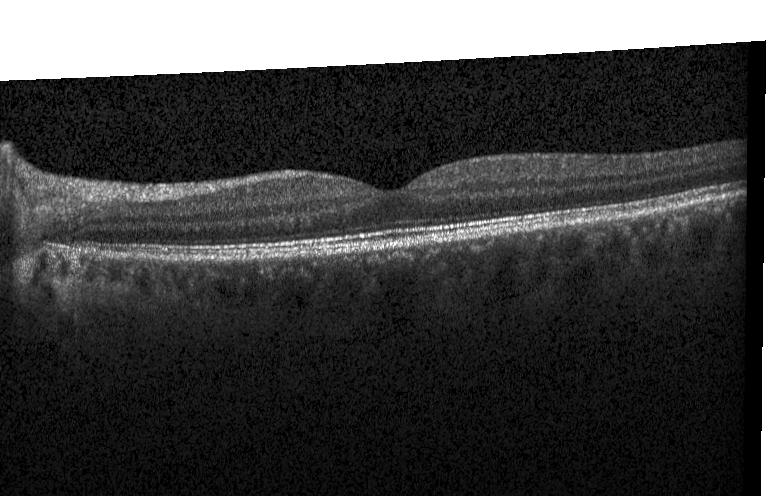 Heidelberg Spectralis OCT system, SD-OCT, optical coherence tomography scan
Diagnosis: no evidence of choroidal neovascularization, diabetic macular edema, or drusen.